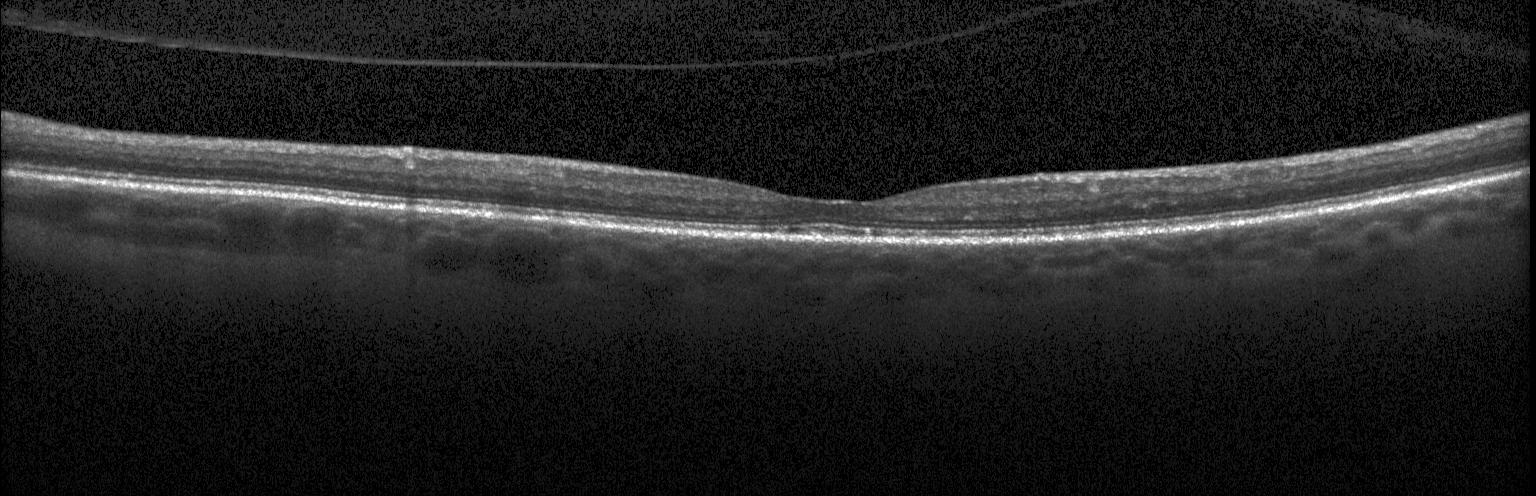 Acquired on a Heidelberg Spectralis. Centered on the fovea. Spectral-domain optical coherence tomography. Optical coherence tomography scan.
OCT finding: no evidence of CNV, DME, or drusen.